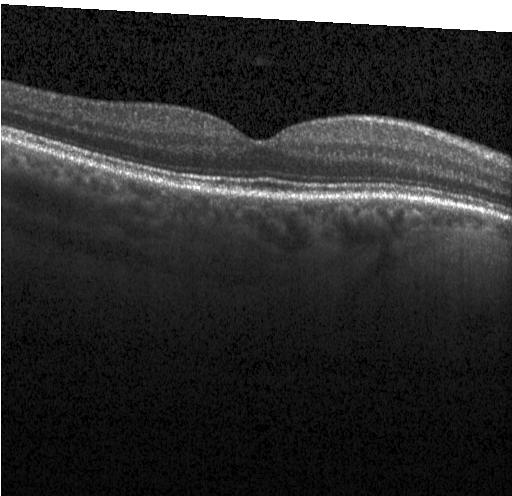
OCT line scan — Assessment: no choroidal neovascularization, diabetic macular edema, or drusen.